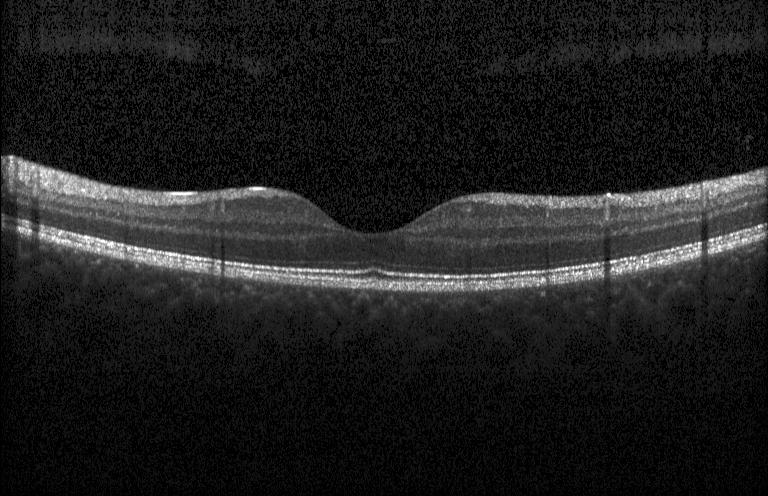
SD-OCT, retinal OCT B-scan
No CNV, no DME, and no drusen.